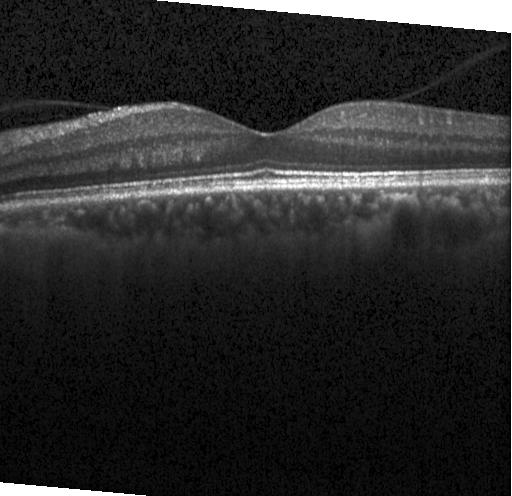
Impression: neither choroidal neovascularization, diabetic macular edema, nor drusen.